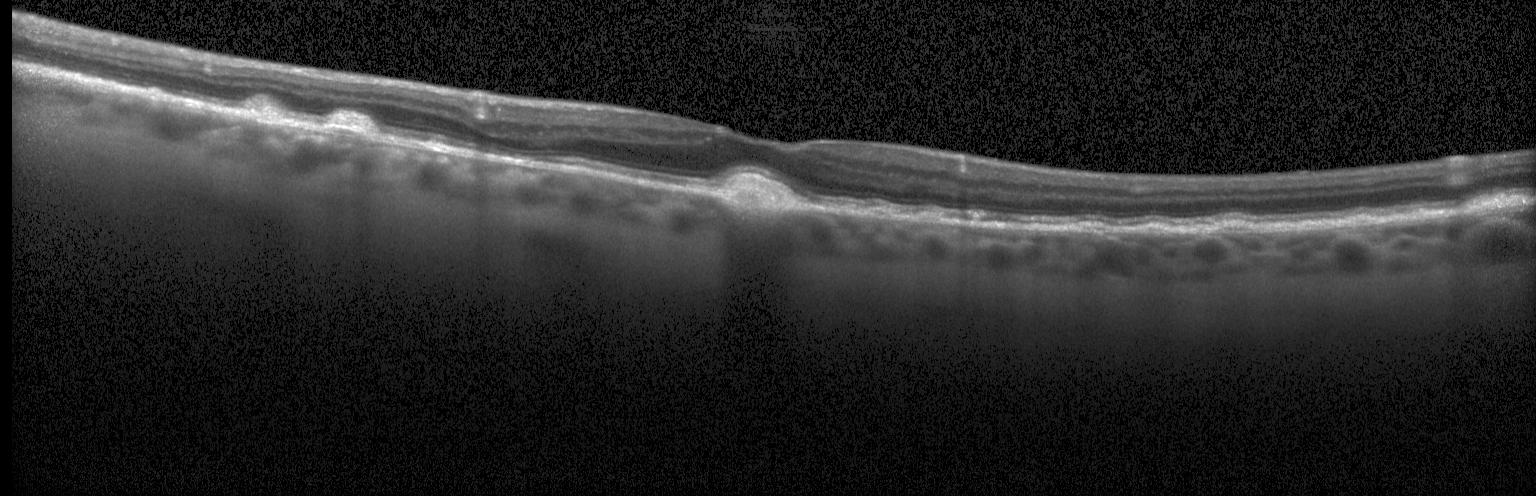

Optical coherence tomography B-scan. Diagnosis: multiple drusen.